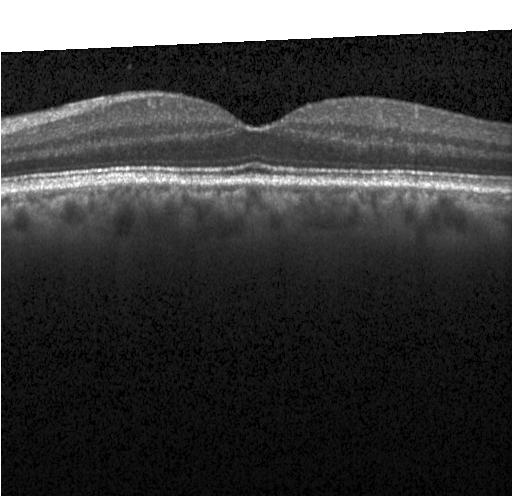

Through the macula, retinal OCT cross-section, spectral-domain optical coherence tomography
Diagnosis: neither CNV, DME, nor drusen.